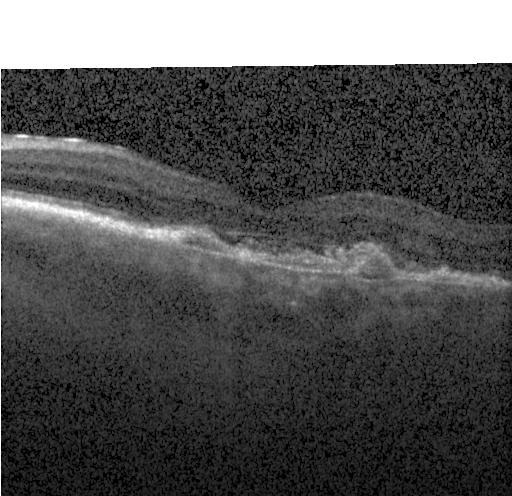
OCT scan showing a choroidal neovascular membrane.